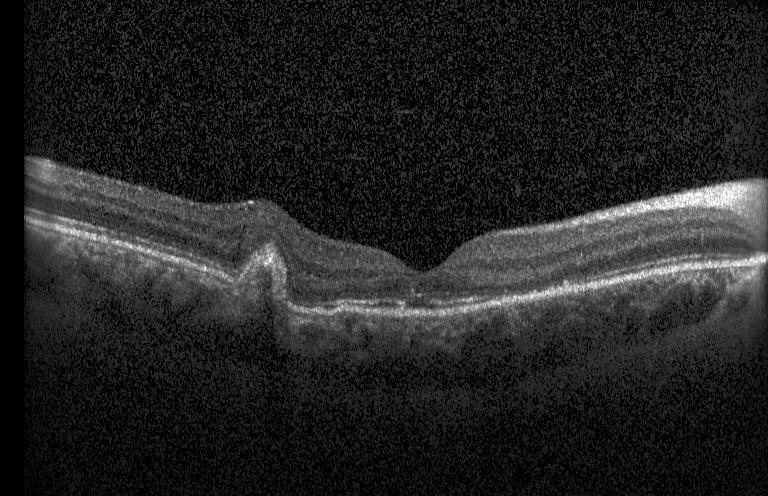

Diagnosis: a choroidal neovascular membrane.